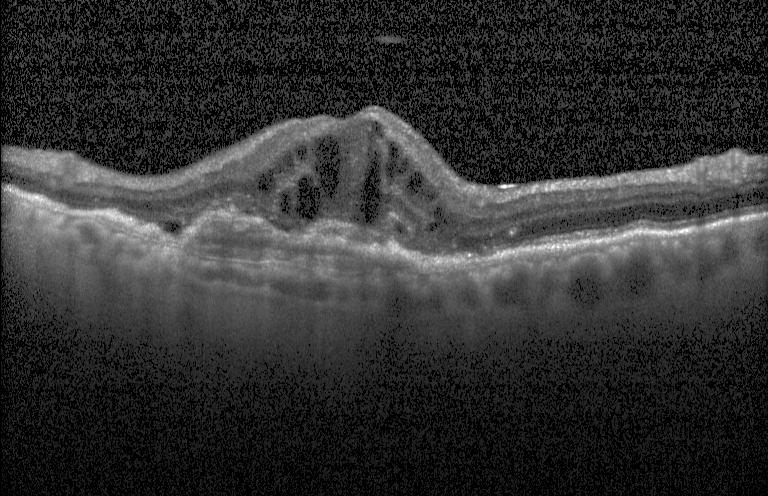
Spectral-domain optical coherence tomography, optical coherence tomography B-scan.
Finding: CNV.